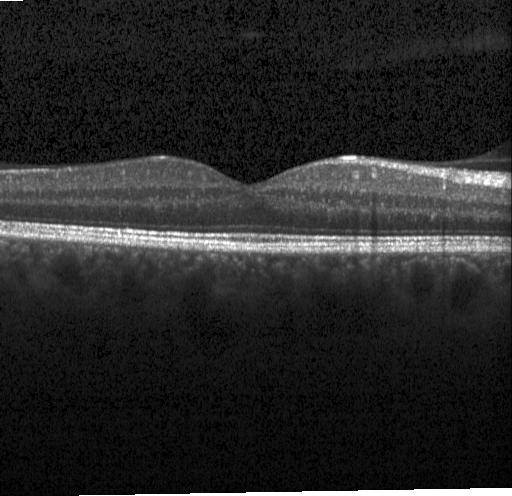 OCT line scan, acquired on a Heidelberg Spectralis, spectral-domain OCT
Impression: neither CNV, DME, nor drusen.